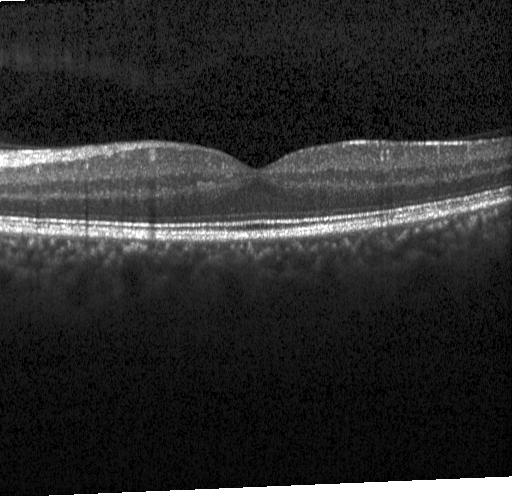

OCT scan showing no evidence of choroidal neovascularization, diabetic macular edema, or drusen.